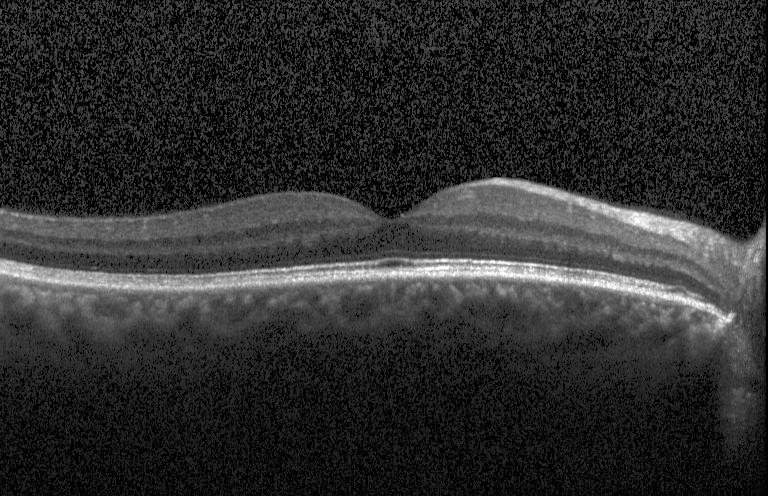
The scan shows no choroidal neovascularization, no diabetic macular edema, and no drusen.